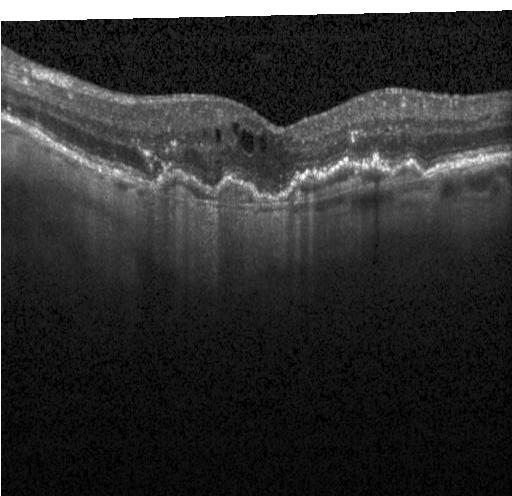

Retinal OCT cross-section; acquired on a Heidelberg Spectralis; macular scan; spectral-domain OCT — The scan shows choroidal neovascularization.